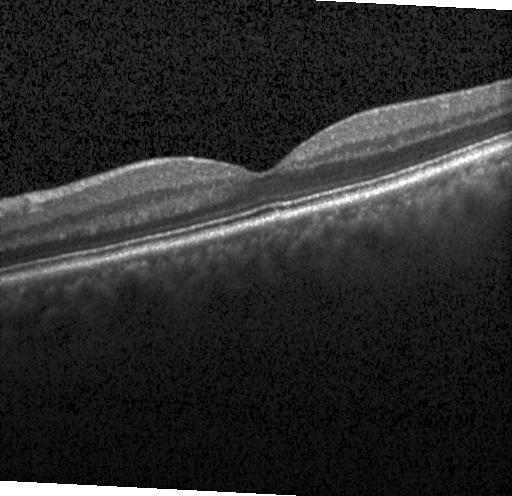
Through the macula · retinal OCT B-scan.
Impression: no CNV, DME, or drusen.